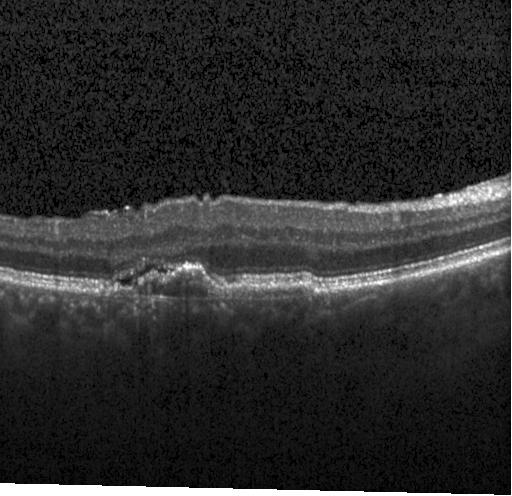

Diagnosis: choroidal neovascularization.